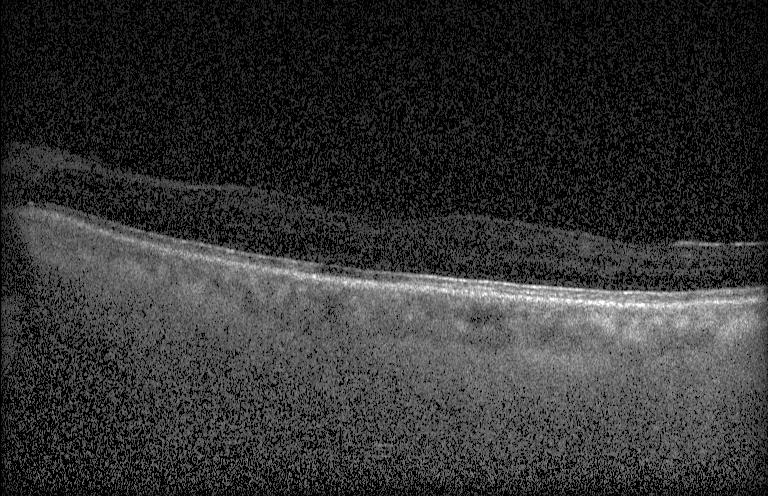
Optical coherence tomography B-scan; instrument: Heidelberg Spectralis — The scan shows no evidence of CNV, DME, or drusen.